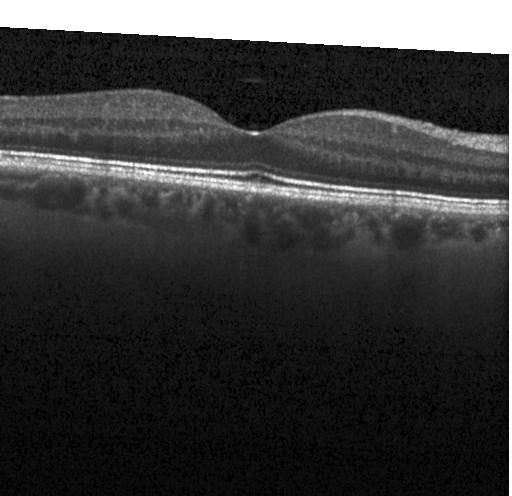 Macular OCT demonstrating no choroidal neovascularization, no diabetic macular edema, and no drusen.